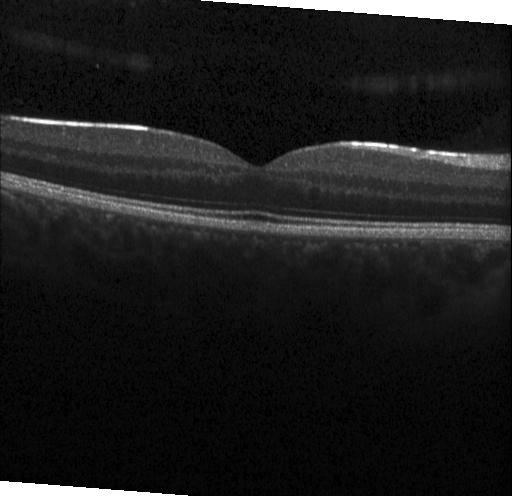
Optical coherence tomography scan
No evidence of CNV, DME, or drusen.